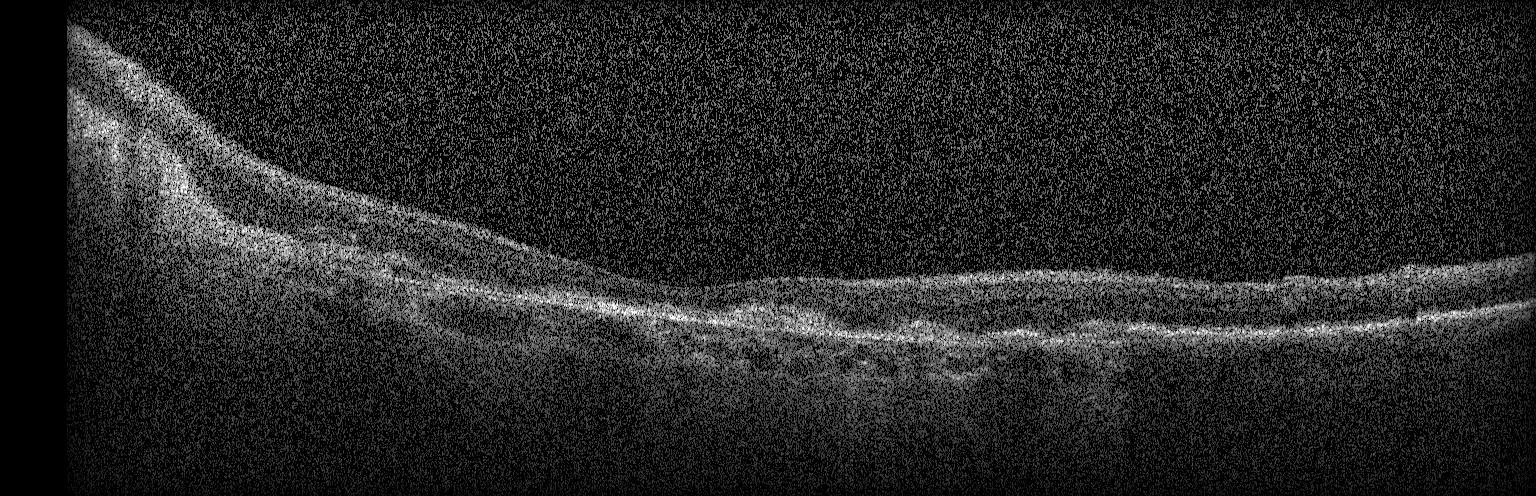
Spectral-domain optical coherence tomography. Acquired on a Heidelberg Spectralis. OCT B-scan. Diagnosis: choroidal neovascularization.